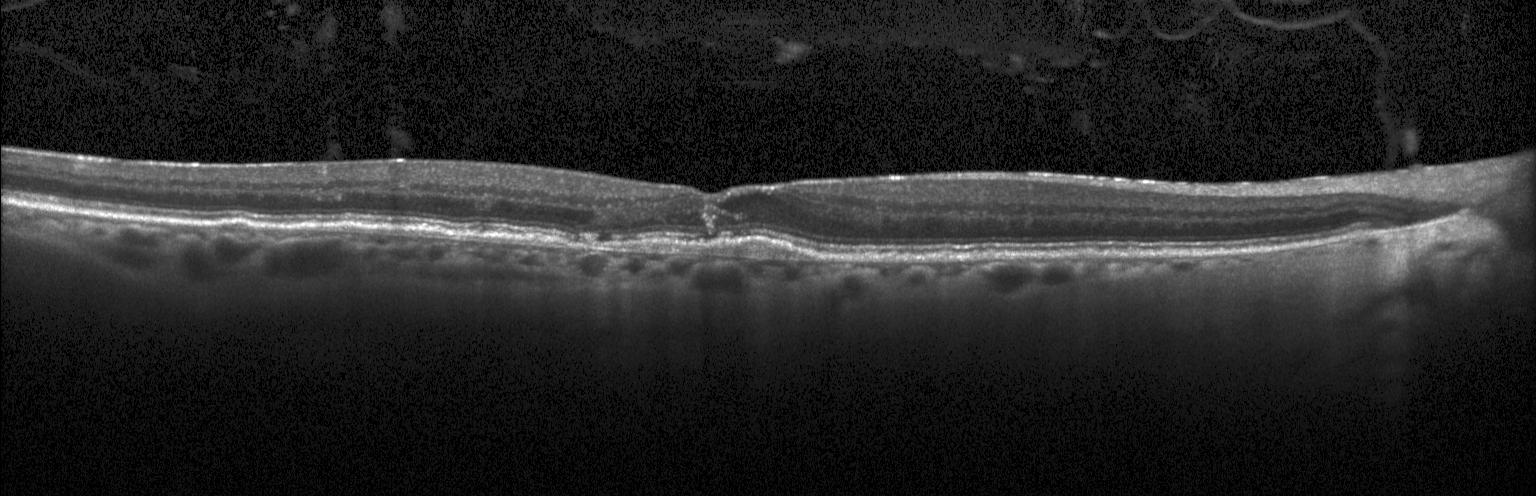 OCT scan showing choroidal neovascularization (CNV).